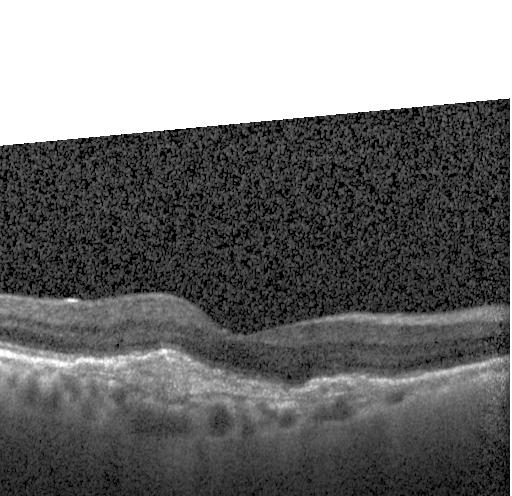
Instrument: Heidelberg Spectralis. Spectral-domain OCT. Retinal OCT cross-section. Centered on the fovea
Macular OCT: a choroidal neovascular membrane.